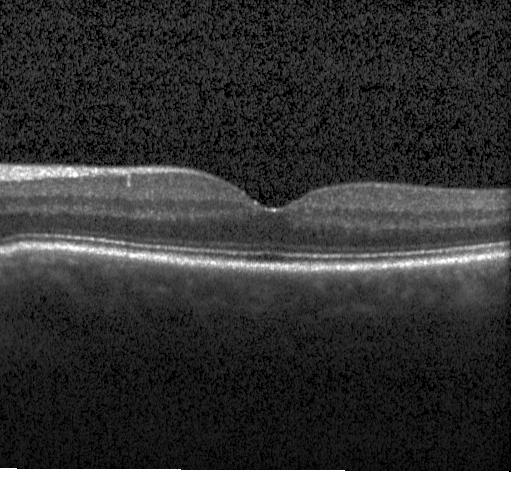
Dx: neither choroidal neovascularization, diabetic macular edema, nor drusen.